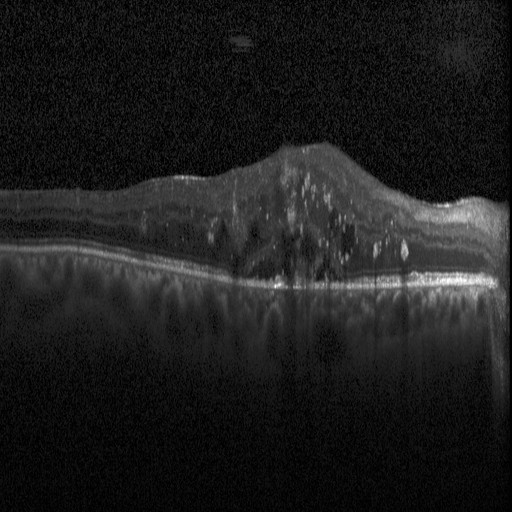
OCT line scan; centered on the fovea
Finding: DME.